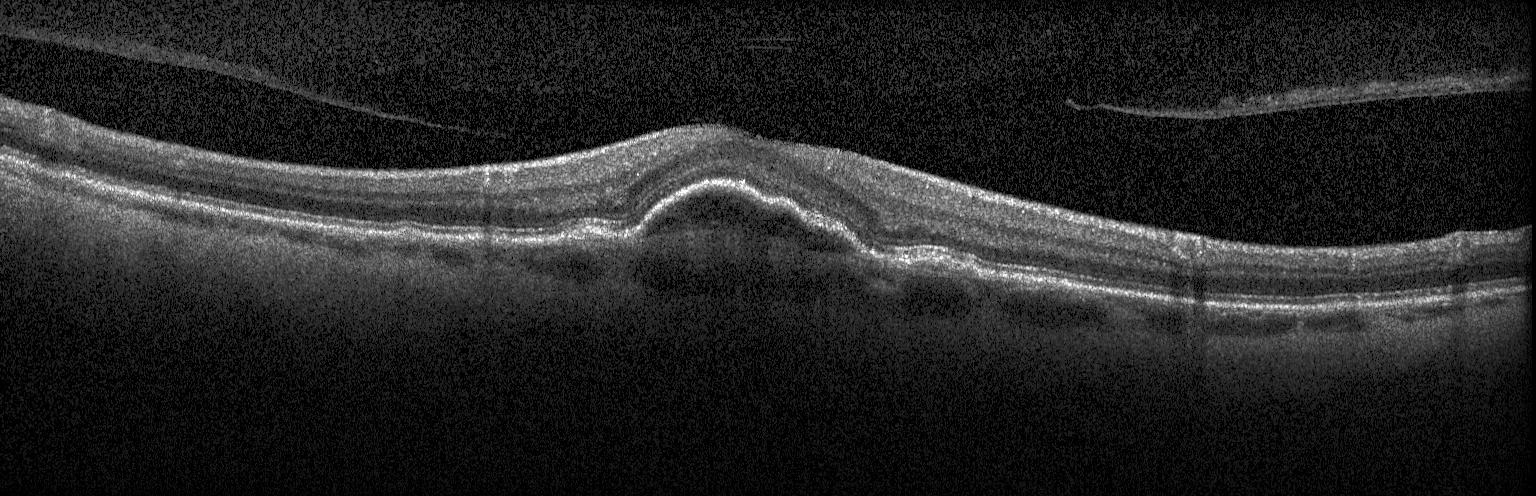 Macular scan; OCT B-scan. Finding: choroidal neovascularization (CNV).